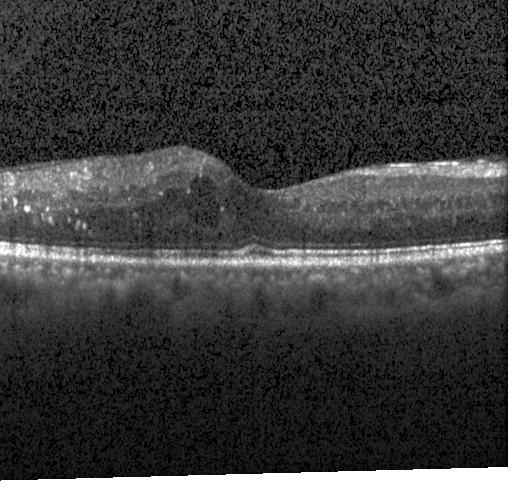
Heidelberg Spectralis OCT system, fovea-centered, OCT B-scan, SD-OCT — DME.